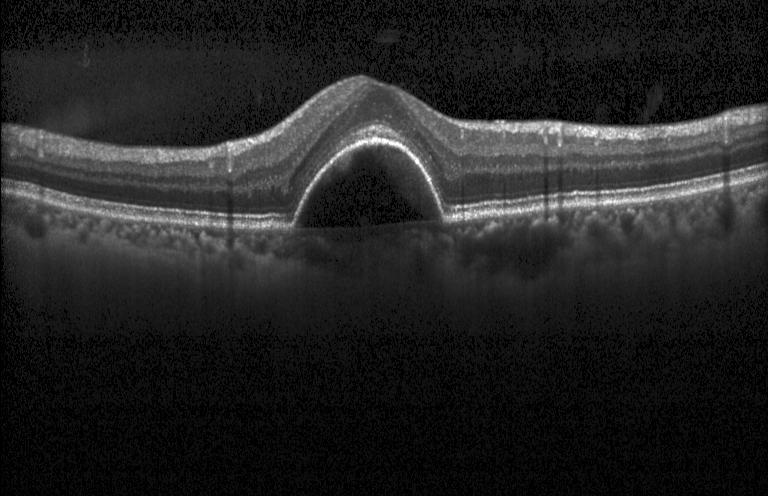

The scan shows a choroidal neovascular membrane.